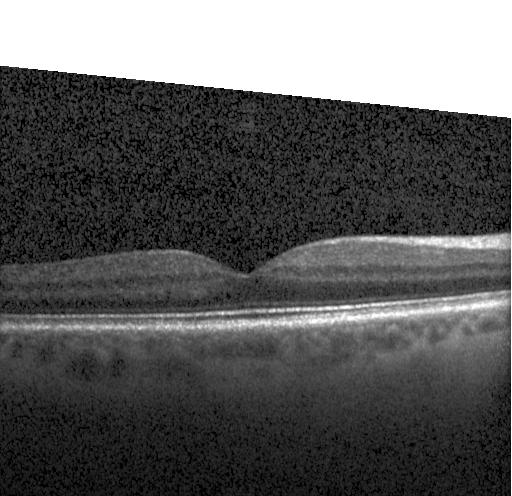

Instrument: Heidelberg Spectralis · spectral-domain OCT · horizontal scan through the fovea · retinal OCT B-scan. This B-scan demonstrates no choroidal neovascularization, diabetic macular edema, or drusen.